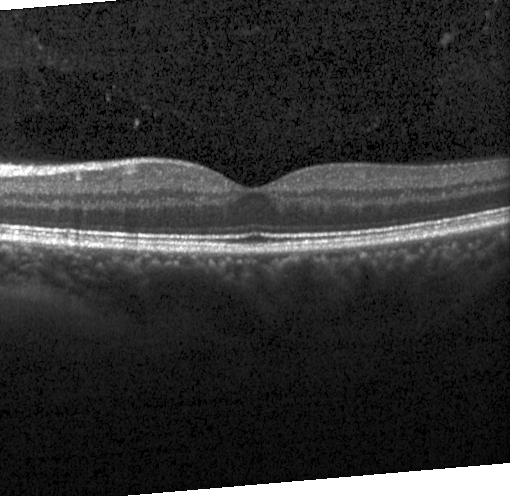

Optical coherence tomography scan; fovea-centered.
Dx: no choroidal neovascularization, no diabetic macular edema, and no drusen.